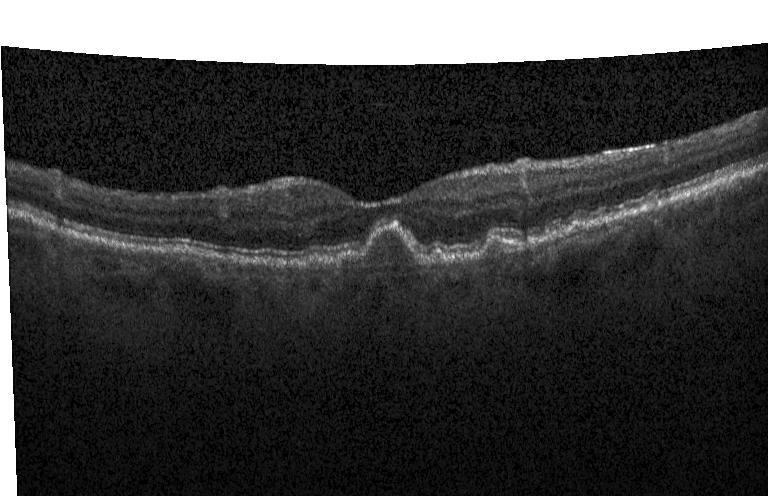 OCT B-scan, SD-OCT.
Diagnosis: sub-RPE drusenoid deposits.